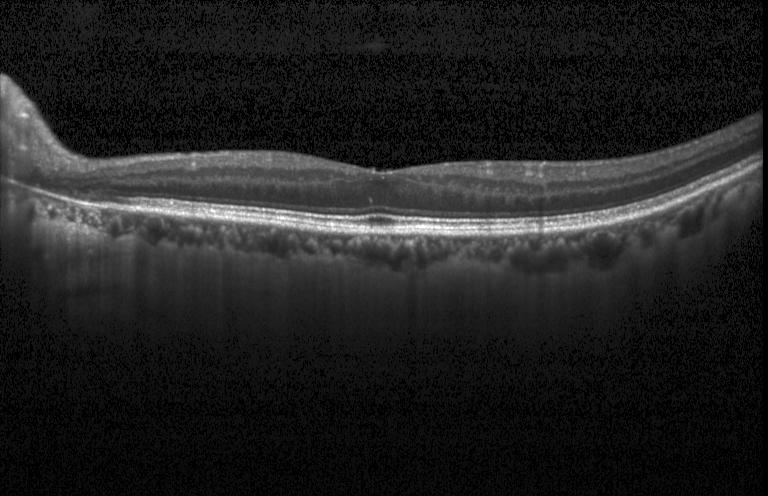 Finding: no evidence of choroidal neovascularization, diabetic macular edema, or drusen.